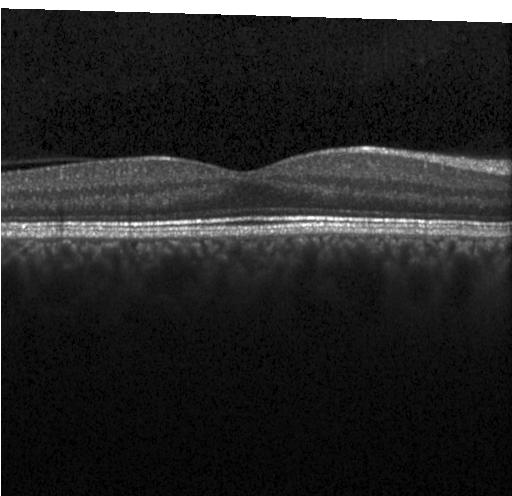
Heidelberg Spectralis. Spectral-domain optical coherence tomography. Optical coherence tomography scan. Horizontal scan through the fovea.
Diagnosis: no CNV, no DME, and no drusen.